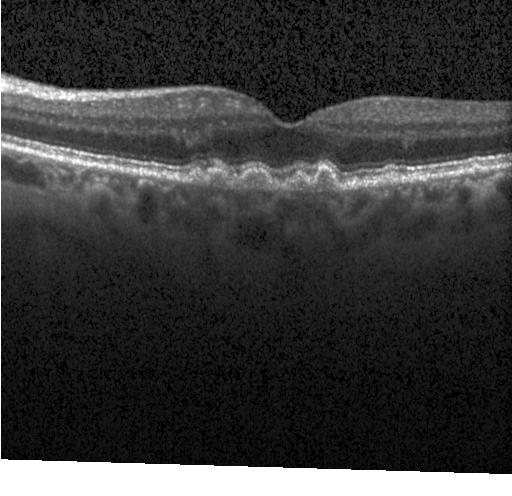 Retinal OCT B-scan; Heidelberg Spectralis OCT system; fovea-centered; spectral-domain OCT
Finding: multiple drusen.